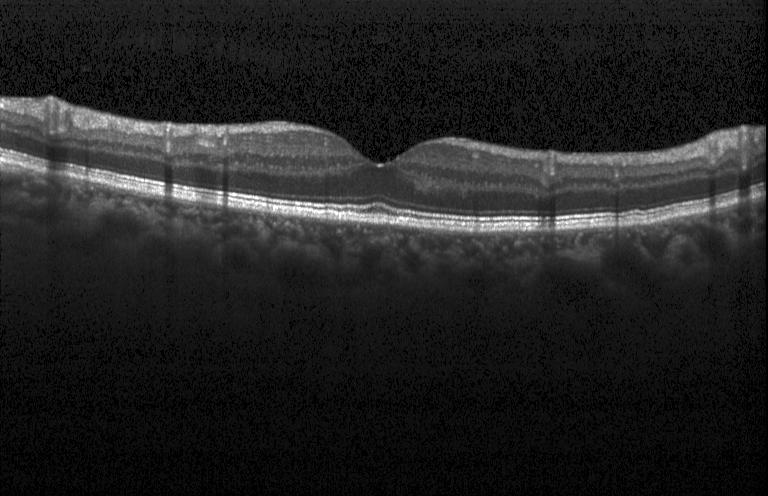
SD-OCT; optical coherence tomography B-scan; Heidelberg Spectralis; macular scan — No choroidal neovascularization, no diabetic macular edema, and no drusen.